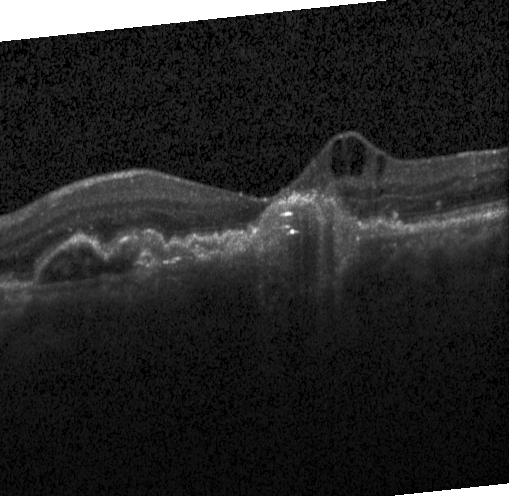 Retinal OCT cross-section. SD-OCT. Acquired on a Heidelberg Spectralis
This B-scan demonstrates CNV.